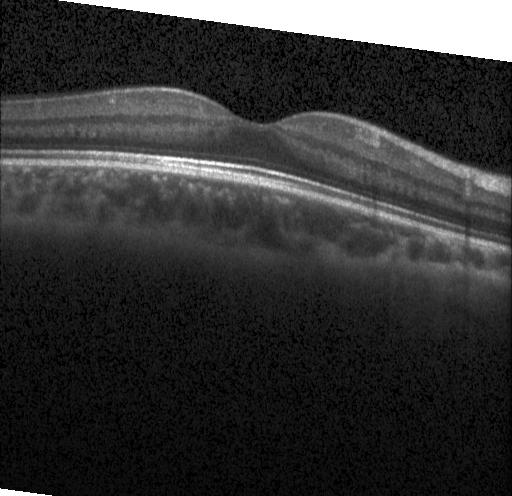

Instrument: Heidelberg Spectralis, SD-OCT, centered on the fovea, retinal OCT B-scan
The scan shows no choroidal neovascularization, no diabetic macular edema, and no drusen.